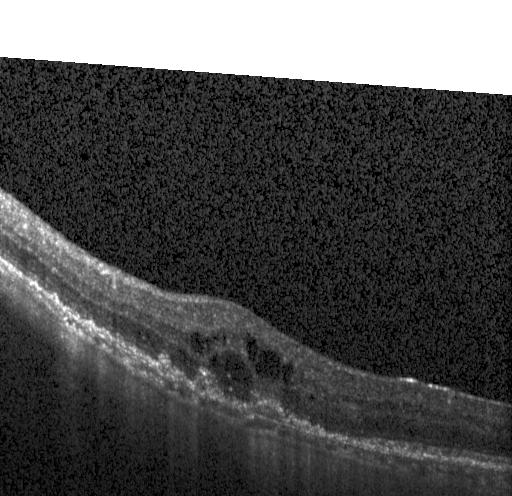
Assessment: a choroidal neovascular membrane.